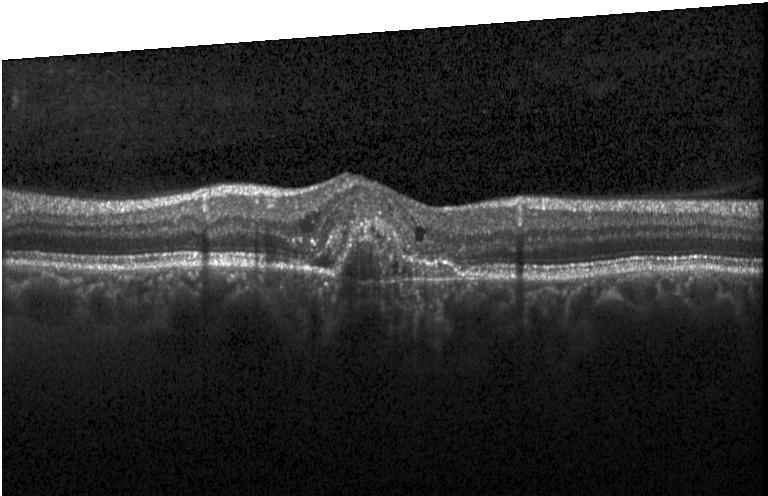

OCT B-scan, fovea-centered, Heidelberg Spectralis, spectral-domain OCT.
Impression: a choroidal neovascular membrane.